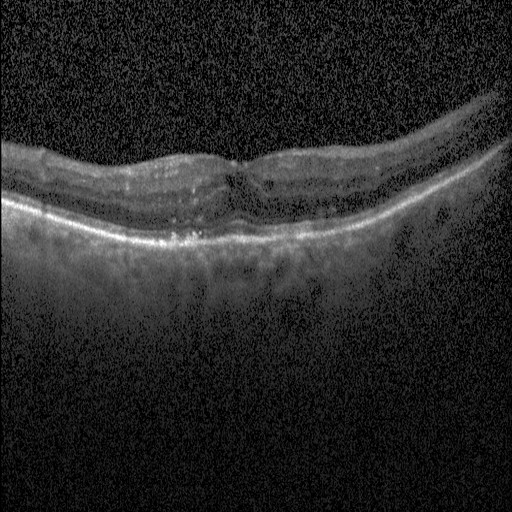

Fovea-centered · OCT B-scan · spectral-domain optical coherence tomography · Heidelberg Spectralis.
Finding: DME.